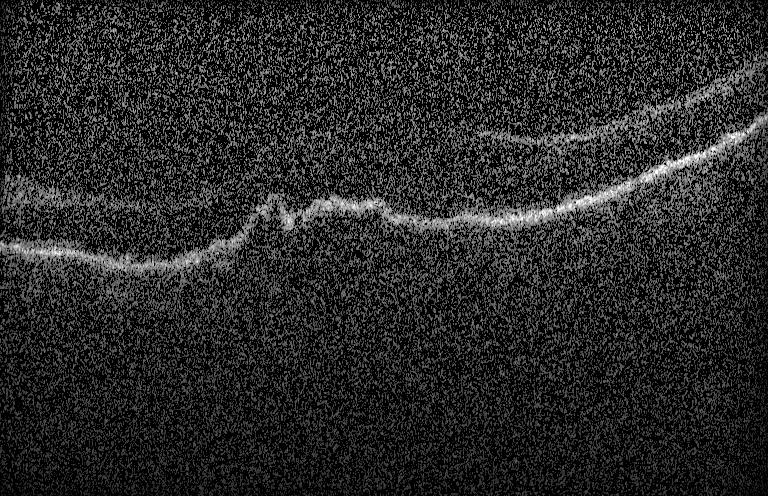 Heidelberg Spectralis. Fovea-centered. OCT B-scan. SD-OCT. Impression: choroidal neovascularization (CNV).